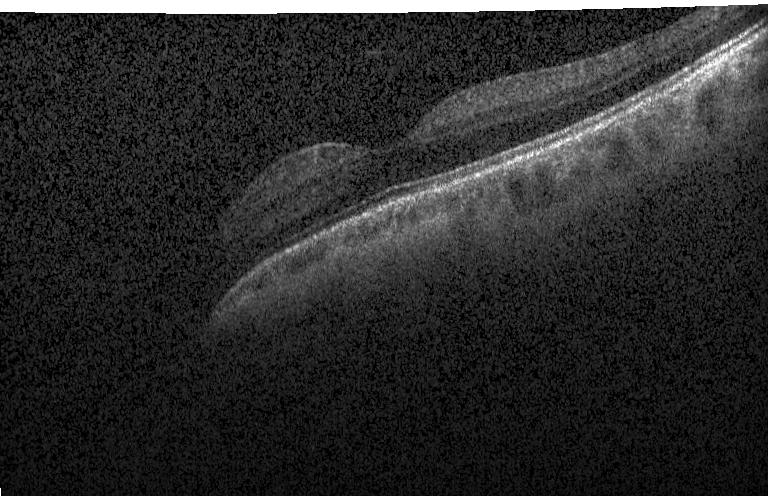

Optical coherence tomography B-scan
Diagnosis: no CNV, no DME, and no drusen.